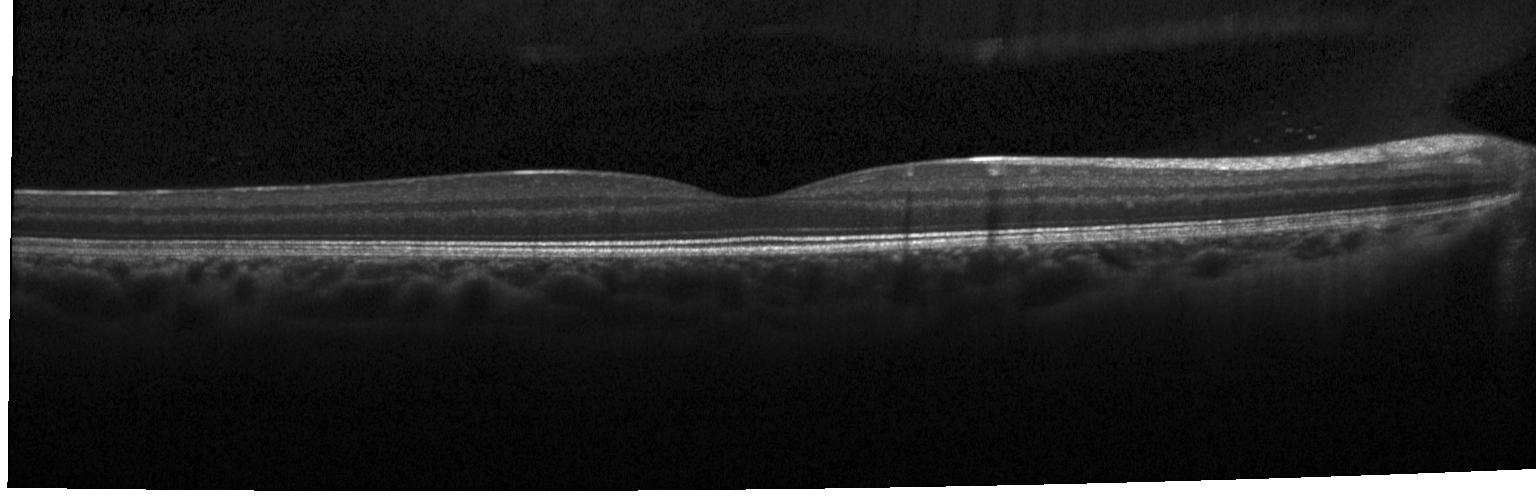
This B-scan demonstrates no CNV, DME, or drusen.